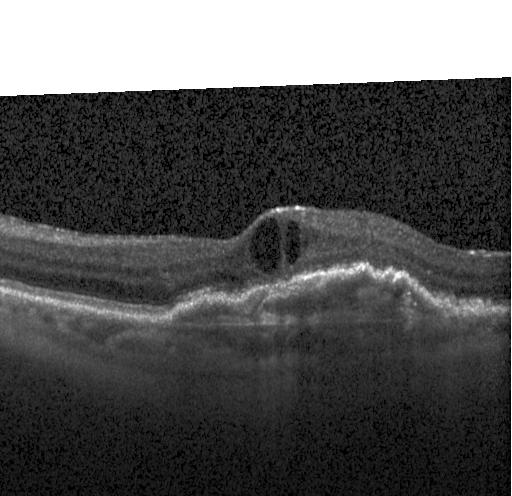
Macular OCT: choroidal neovascularization.